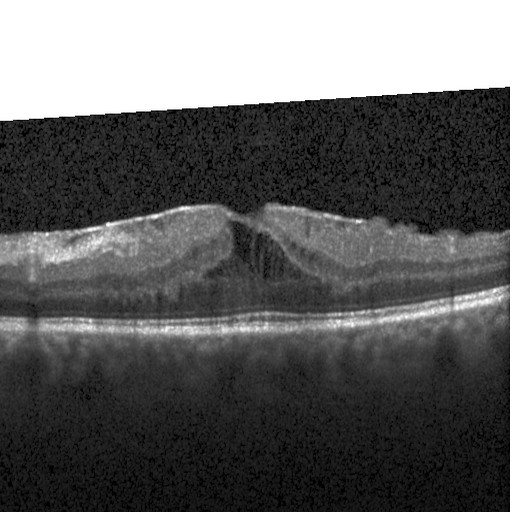
Centered on the fovea. Optical coherence tomography scan. Acquired on a Heidelberg Spectralis
DME.